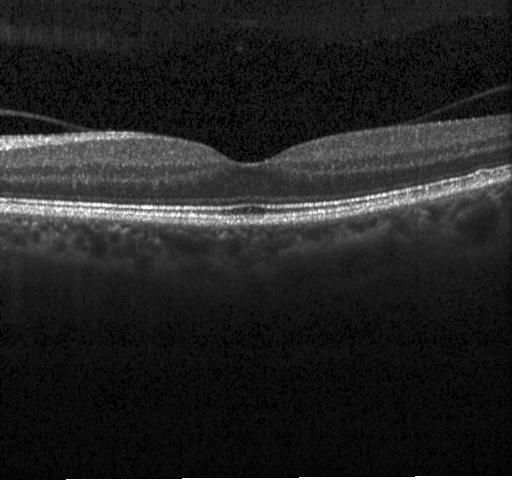 Optical coherence tomography B-scan; horizontal scan through the fovea
Diagnosis: no choroidal neovascularization, diabetic macular edema, or drusen.